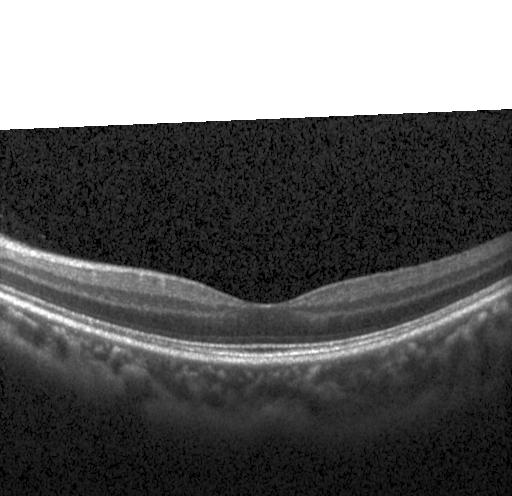

Retinal OCT cross-section · spectral-domain optical coherence tomography · horizontal scan through the fovea · Heidelberg Spectralis OCT system
OCT finding: no choroidal neovascularization, no diabetic macular edema, and no drusen.